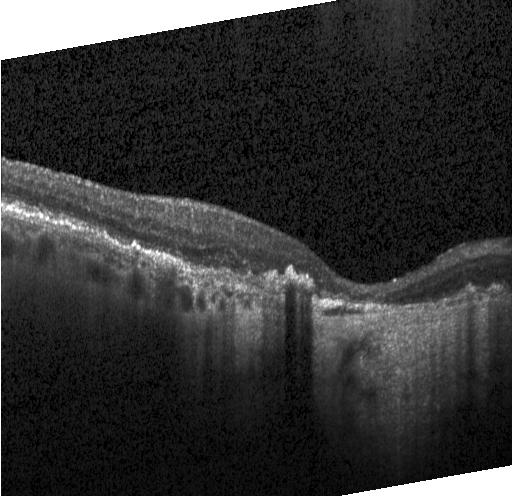
This B-scan demonstrates choroidal neovascularization (CNV).